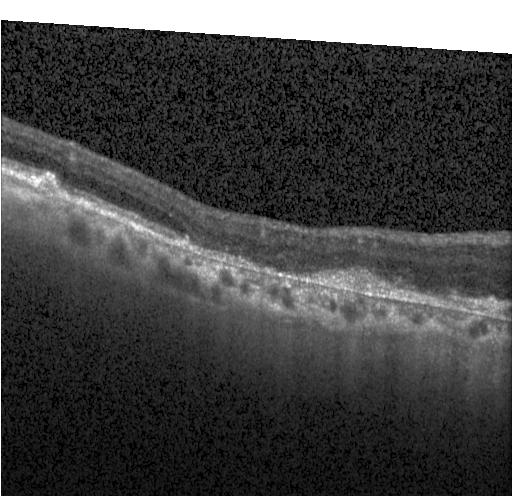

Optical coherence tomography B-scan · macular scan.
Dx: CNV.